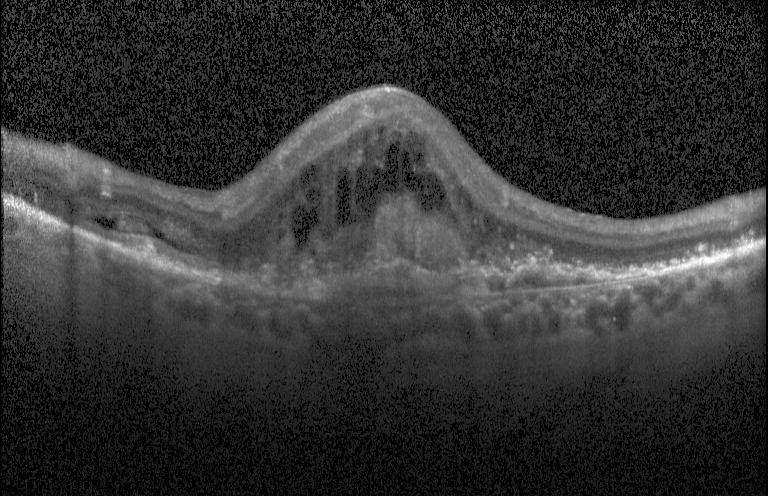

Retinal OCT cross-section · Heidelberg Spectralis OCT system. Assessment: a choroidal neovascular membrane.